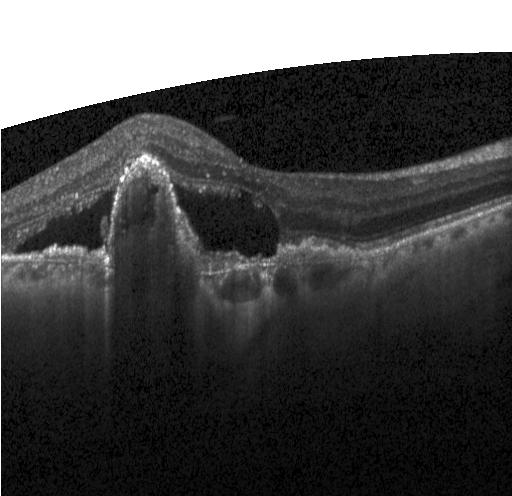 Macular OCT demonstrating a choroidal neovascular membrane.